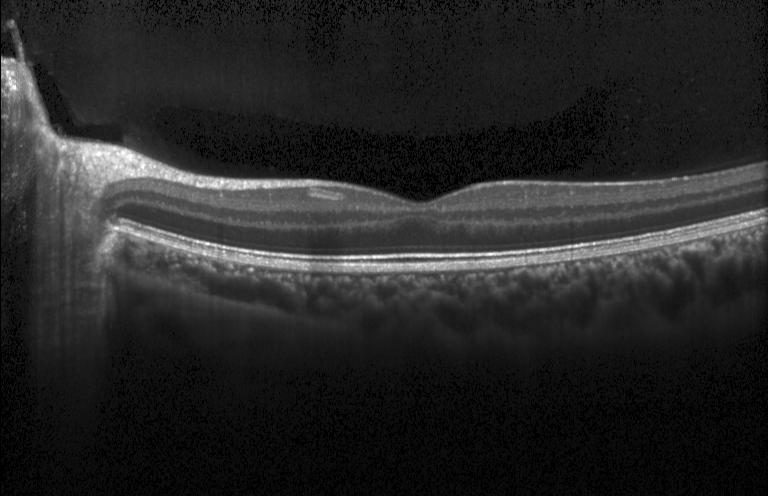 Finding: neither choroidal neovascularization, diabetic macular edema, nor drusen.